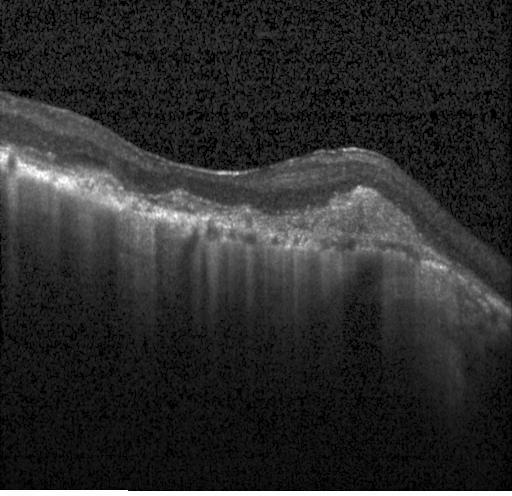
Spectral-domain optical coherence tomography · through the macula · acquired on a Heidelberg Spectralis · OCT line scan
Macular OCT: a choroidal neovascular membrane.